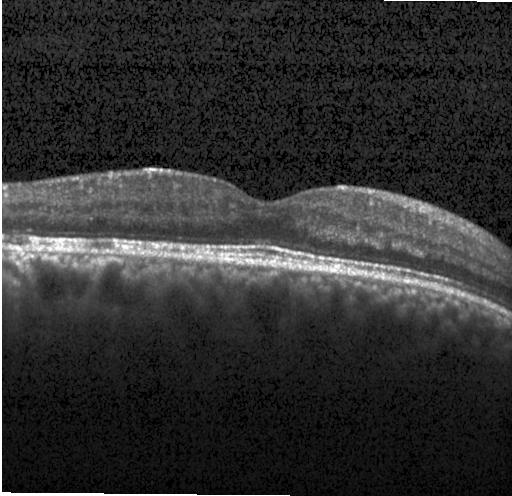 OCT B-scan. Spectral-domain OCT. Through the macula. Instrument: Heidelberg Spectralis. Assessment: no evidence of choroidal neovascularization, diabetic macular edema, or drusen.